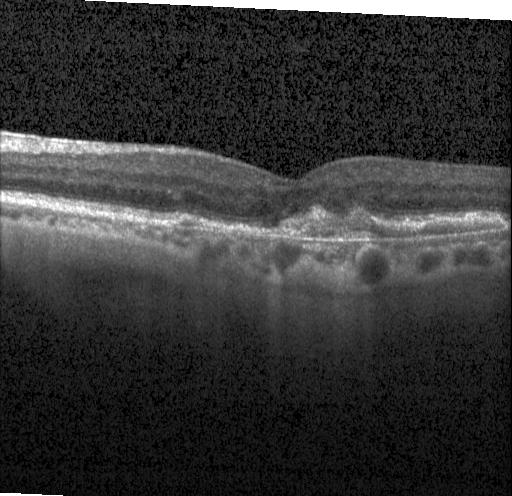

Impression: choroidal neovascularization (CNV).